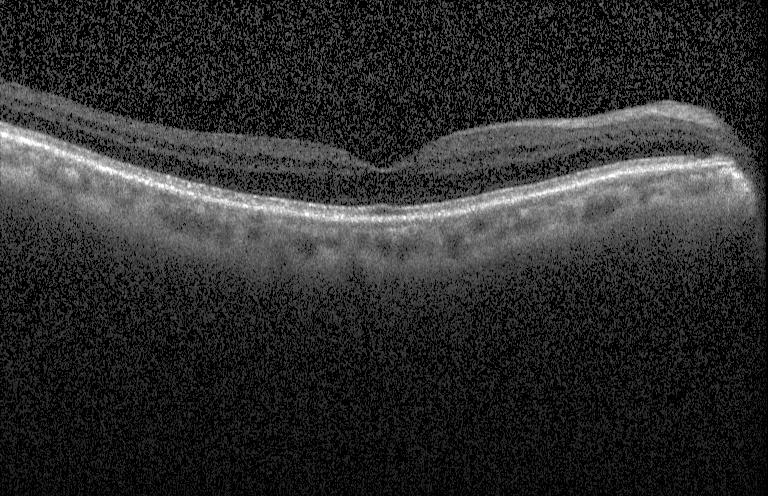

Heidelberg Spectralis OCT system, OCT line scan — OCT finding: no choroidal neovascularization, diabetic macular edema, or drusen.